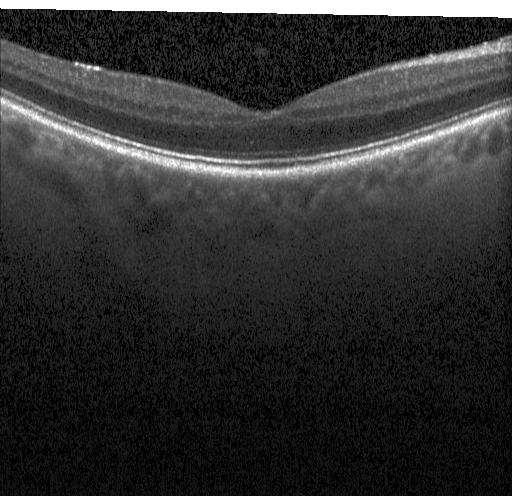 Spectral-domain OCT; OCT line scan; acquired on a Heidelberg Spectralis
Impression: no evidence of choroidal neovascularization, diabetic macular edema, or drusen.